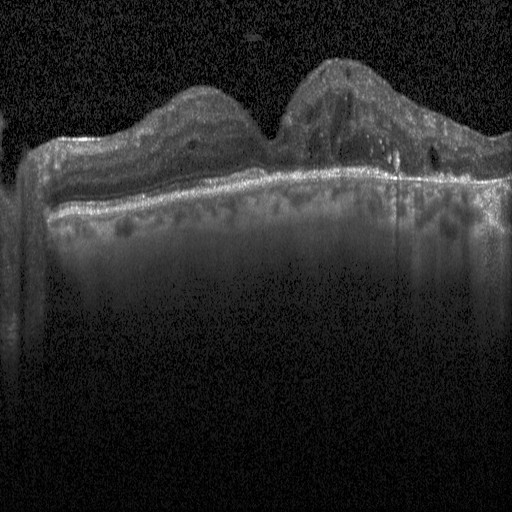
OCT line scan — Macular OCT: diabetic macular edema (DME).